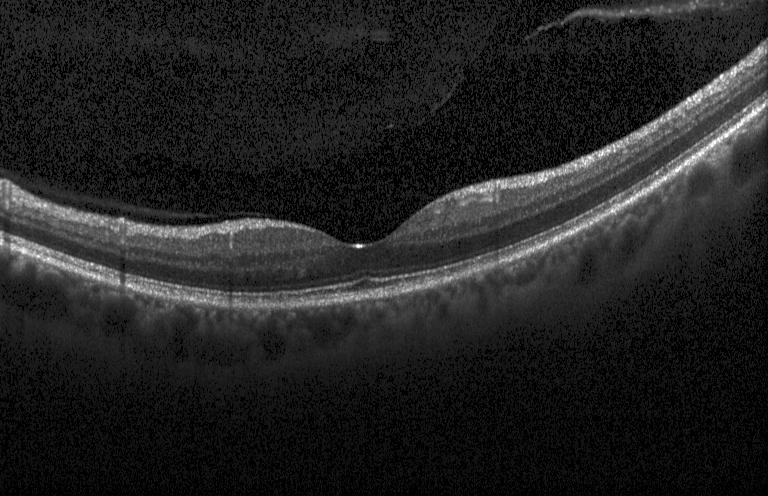 Diagnosis: no CNV, no DME, and no drusen.